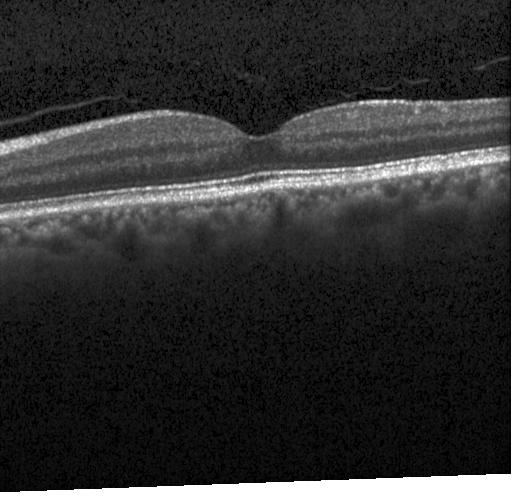
Retinal OCT cross-section showing no CNV, DME, or drusen.